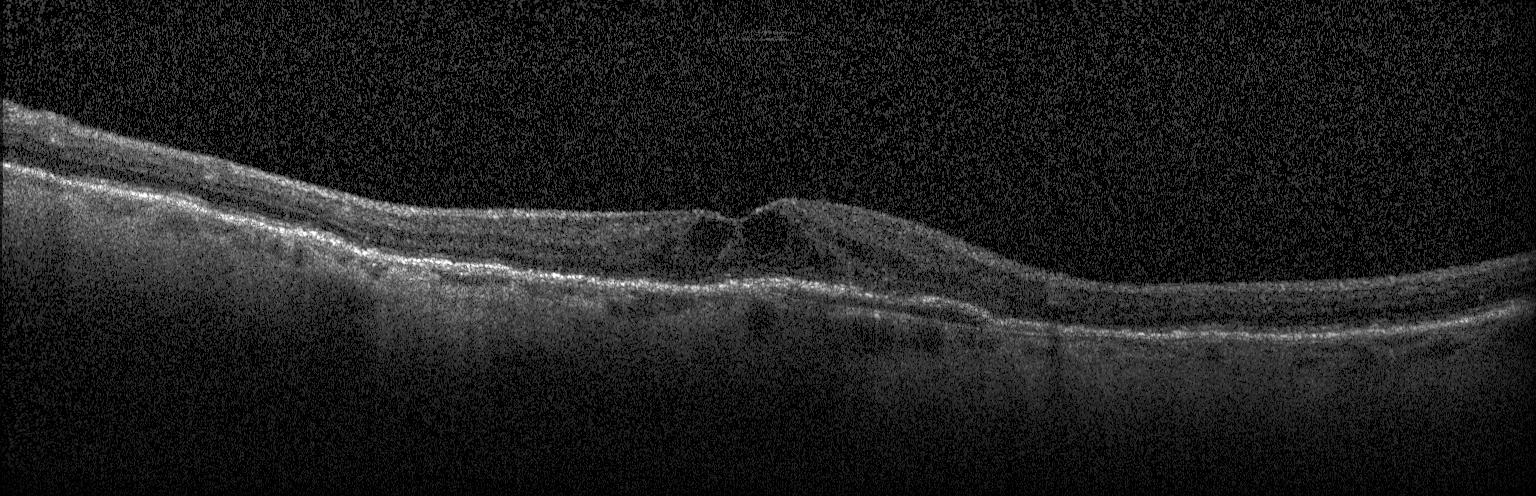 Heidelberg Spectralis; through the macula; optical coherence tomography B-scan
Impression: a choroidal neovascular membrane.